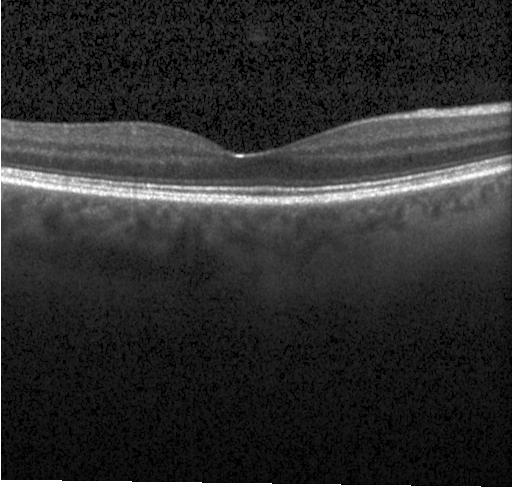
Optical coherence tomography B-scan; horizontal scan through the fovea
Dx: neither choroidal neovascularization, diabetic macular edema, nor drusen.